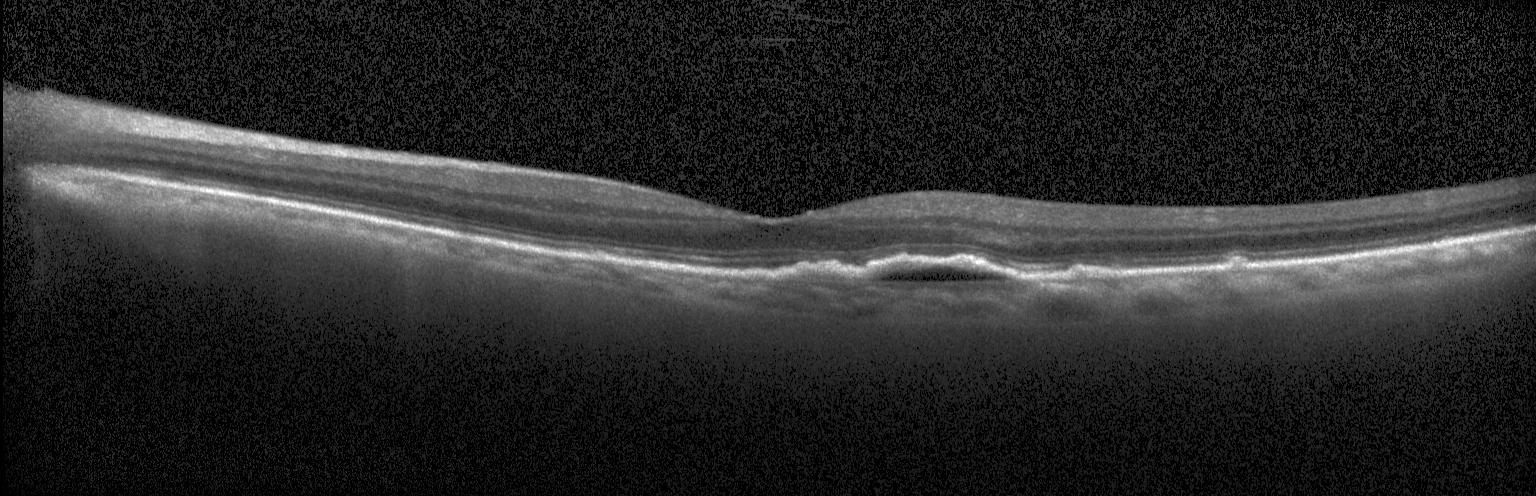

Assessment: a choroidal neovascular membrane.